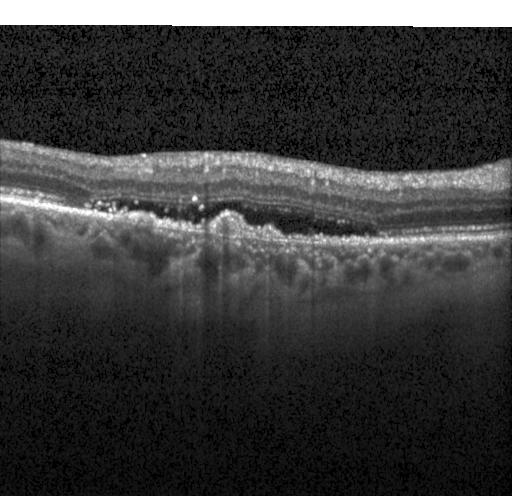 Retinal OCT B-scan, acquired on a Heidelberg Spectralis. The scan shows choroidal neovascularization (CNV).